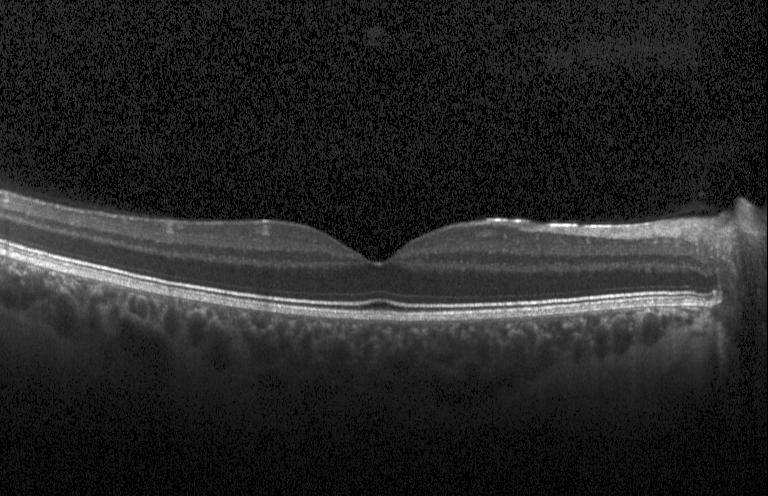

Optical coherence tomography B-scan · through the macula.
Diagnosis: no evidence of choroidal neovascularization, diabetic macular edema, or drusen.